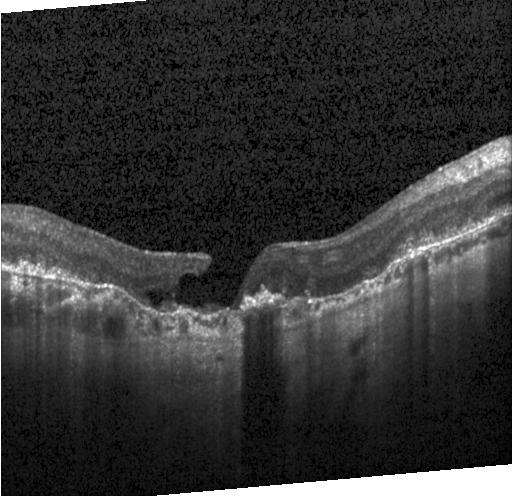 OCT B-scan
A choroidal neovascular membrane.